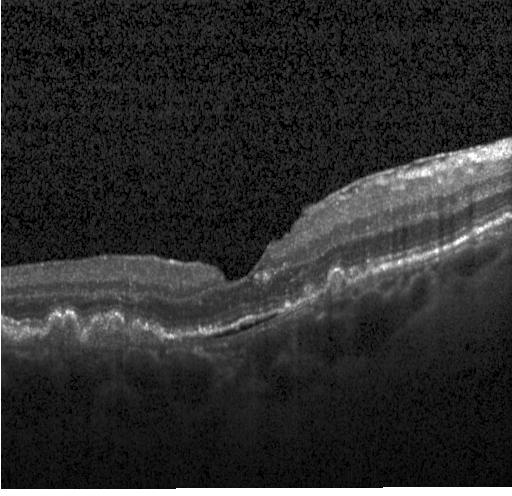

Optical coherence tomography scan; through the macula; spectral-domain optical coherence tomography — Diagnosis: a choroidal neovascular membrane.